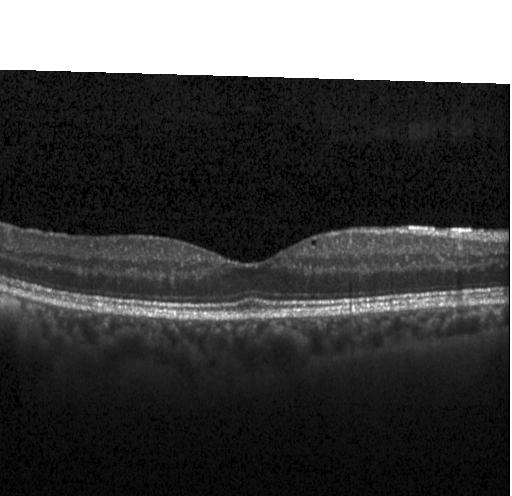

Retinal OCT cross-section, SD-OCT, centered on the fovea, instrument: Heidelberg Spectralis.
Impression: no choroidal neovascularization, no diabetic macular edema, and no drusen.